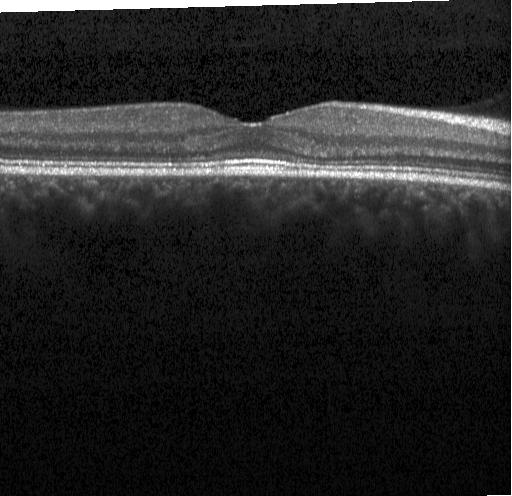
No CNV, DME, or drusen.